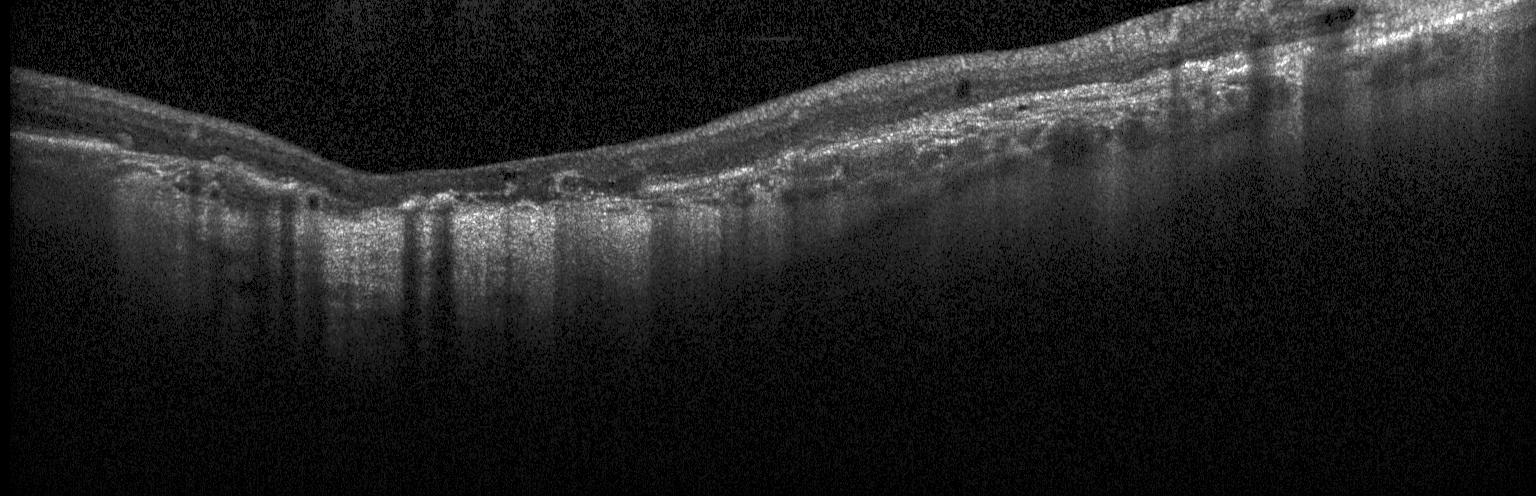 SD-OCT · optical coherence tomography scan · macular scan — Dx: a choroidal neovascular membrane.